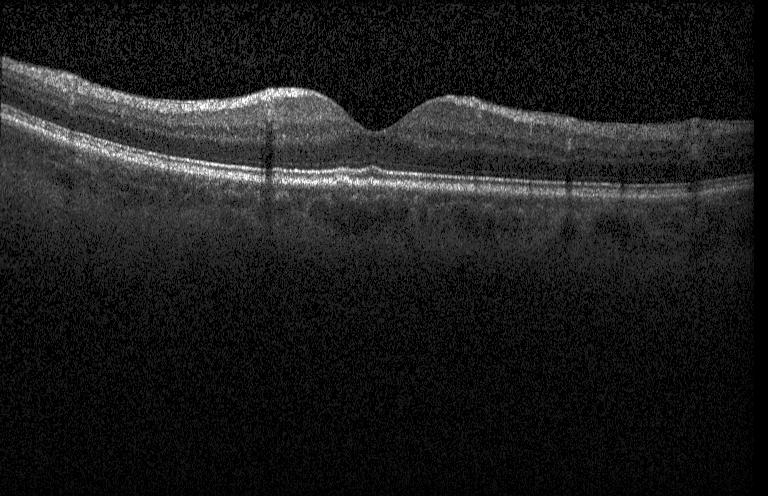

Macular OCT: multiple drusen.